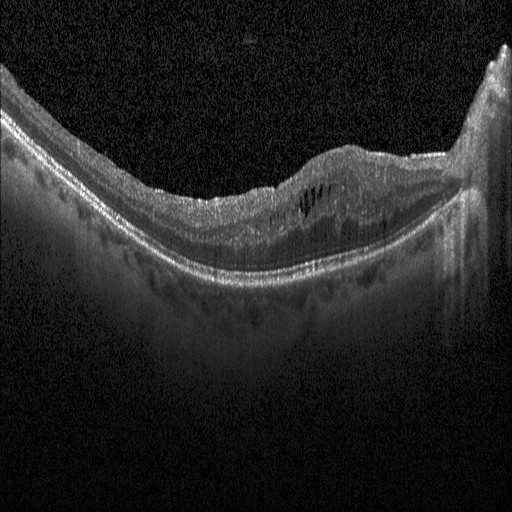
Optical coherence tomography scan.
OCT finding: diabetic macular edema.